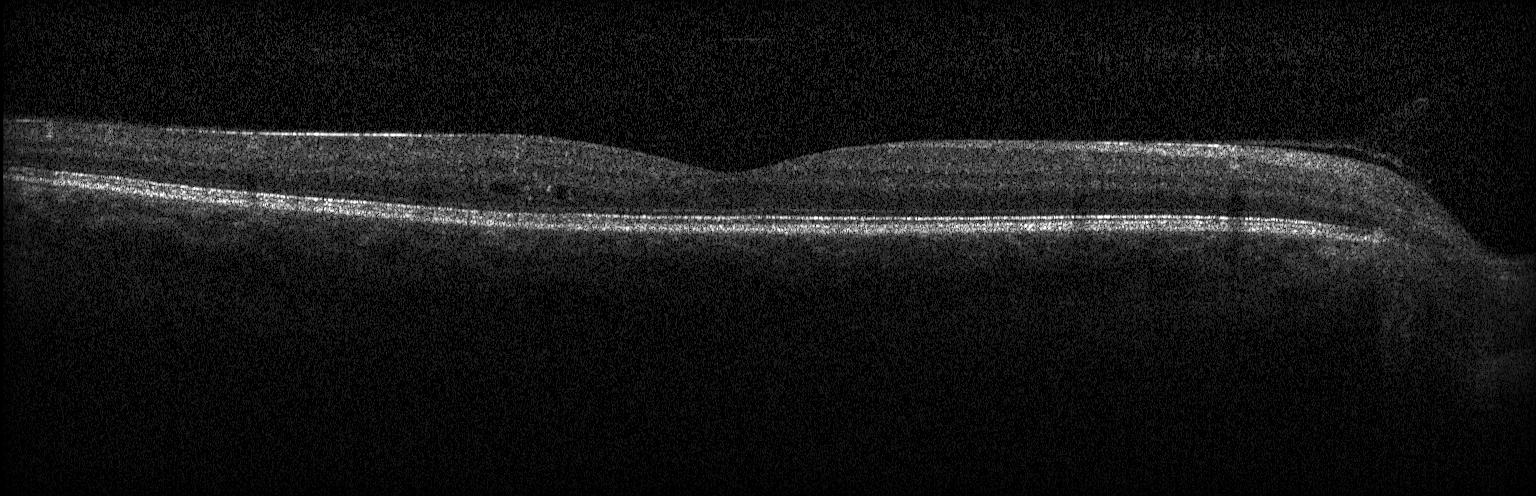 Retinal OCT cross-section — Finding: no evidence of CNV, DME, or drusen.